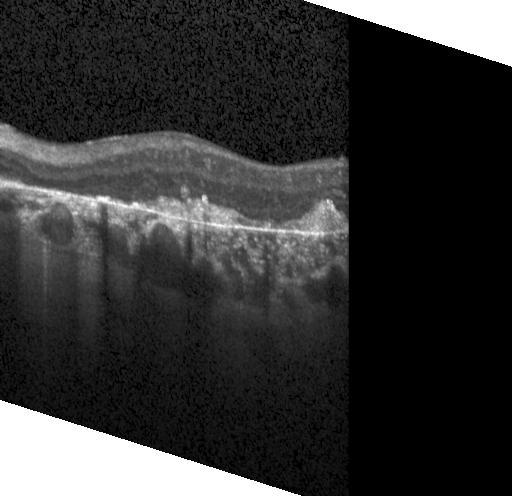

Retinal OCT cross-section; Heidelberg Spectralis OCT system; spectral-domain optical coherence tomography. Finding: choroidal neovascularization.